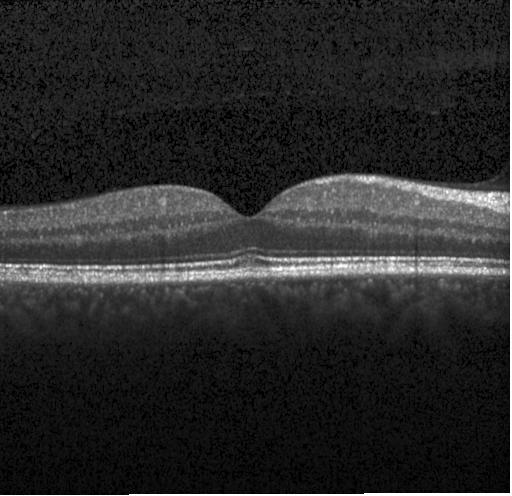 SD-OCT. Optical coherence tomography scan. Acquired on a Heidelberg Spectralis.
The scan shows no choroidal neovascularization, no diabetic macular edema, and no drusen.